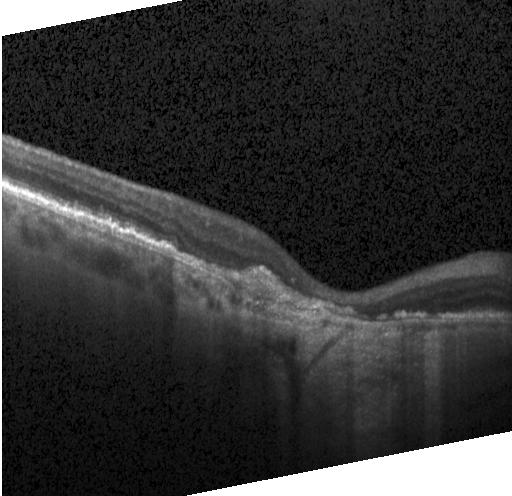
Fovea-centered; retinal OCT cross-section — Assessment: CNV.